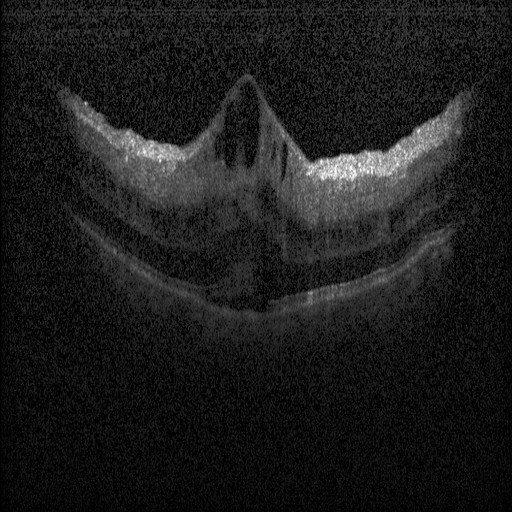
Assessment: DME.